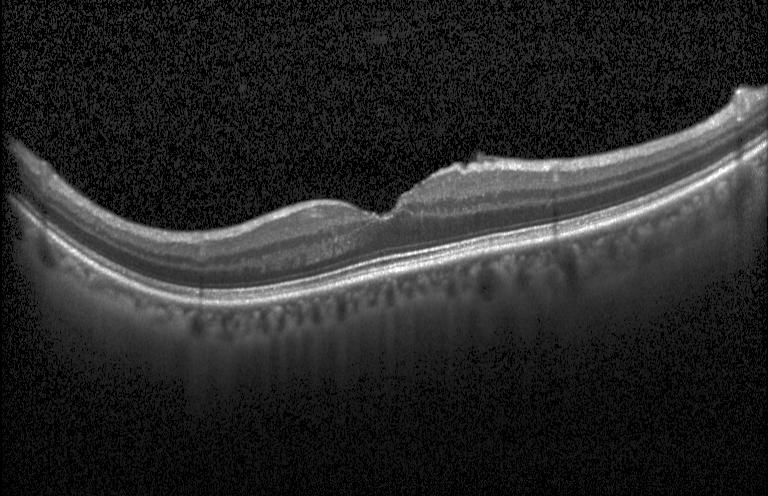 OCT B-scan · fovea-centered · instrument: Heidelberg Spectralis.
Dx: no choroidal neovascularization, diabetic macular edema, or drusen.